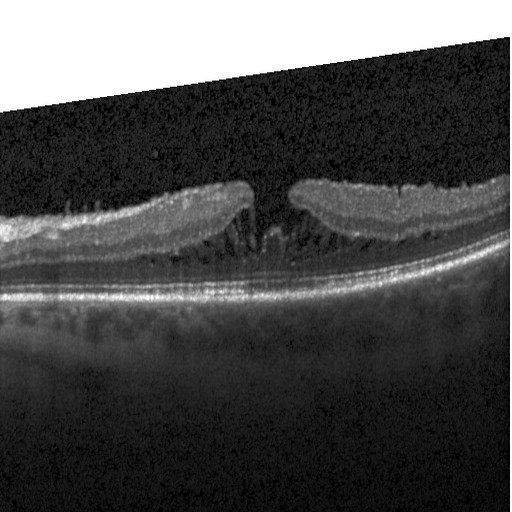 SD-OCT, instrument: Heidelberg Spectralis, centered on the fovea, optical coherence tomography scan — This B-scan demonstrates DME.